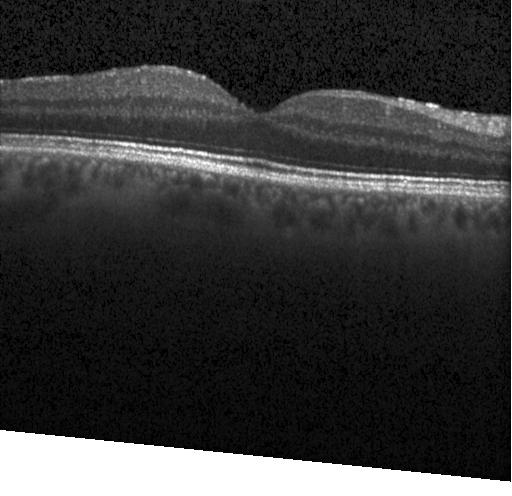

Retinal OCT cross-section
This B-scan demonstrates no evidence of CNV, DME, or drusen.